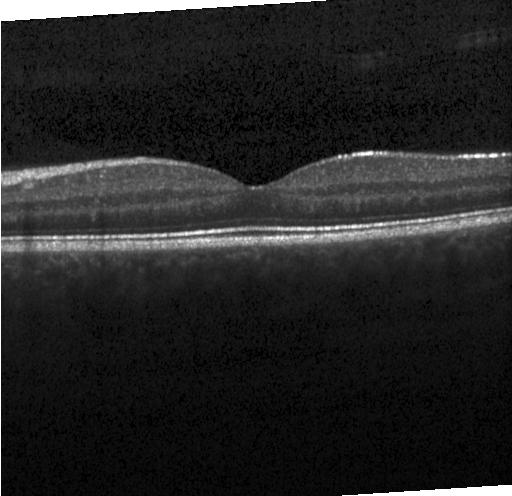 Diagnosis: neither CNV, DME, nor drusen.